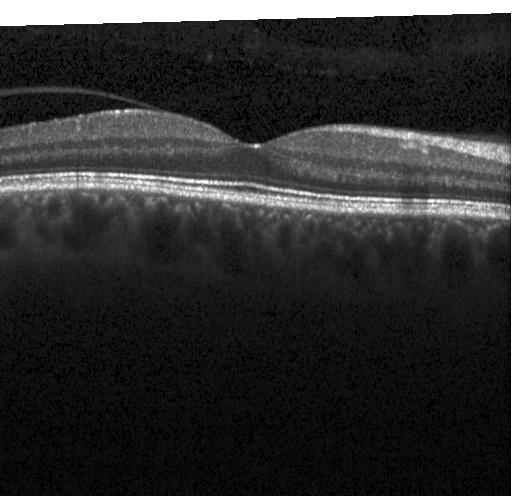

Spectral-domain OCT. Acquired on a Heidelberg Spectralis. Retinal OCT cross-section. Through the macula.
Dx: neither CNV, DME, nor drusen.